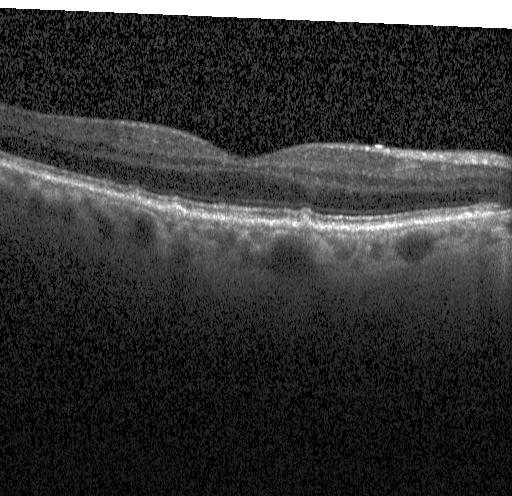

OCT finding: drusen.